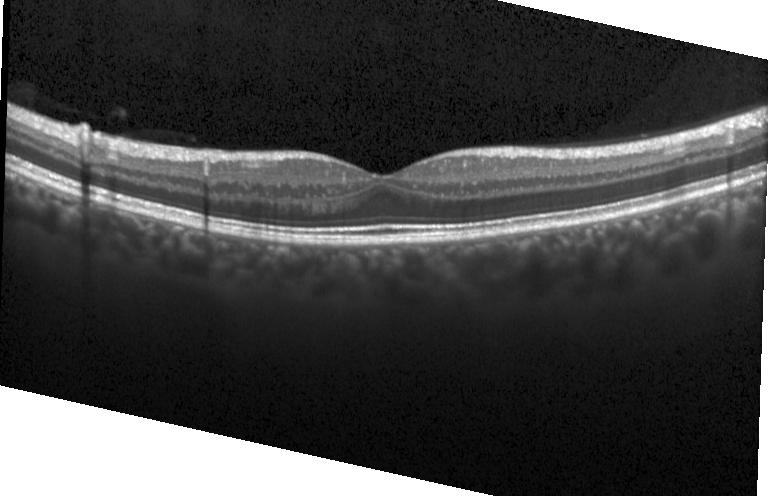
SD-OCT. OCT line scan. Macular OCT: no choroidal neovascularization, diabetic macular edema, or drusen.